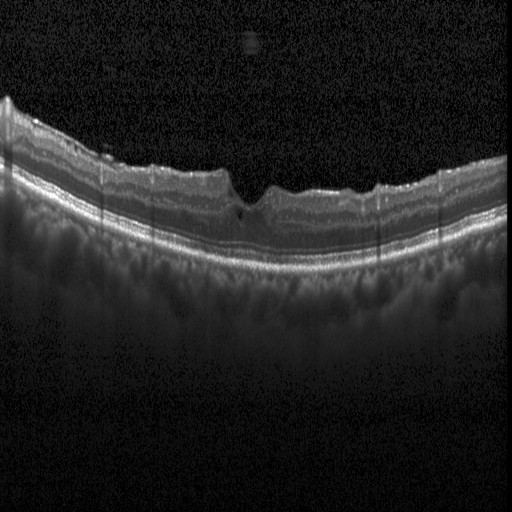
Diabetic macular edema.